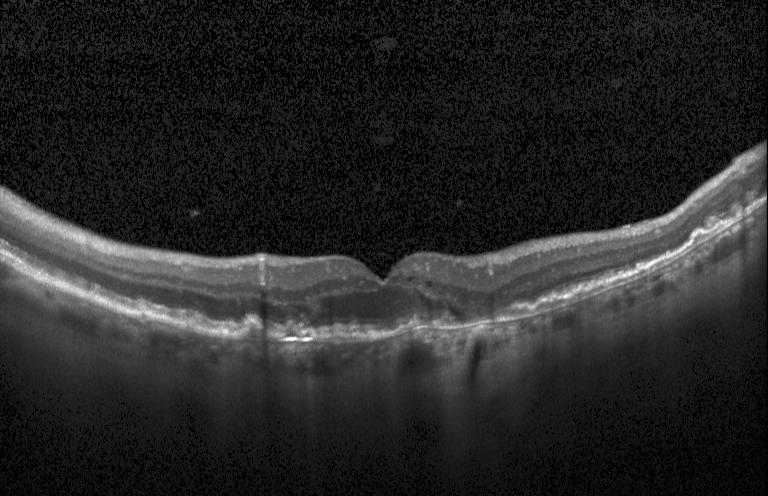 Retinal OCT B-scan, Heidelberg Spectralis OCT system — The scan shows CNV.